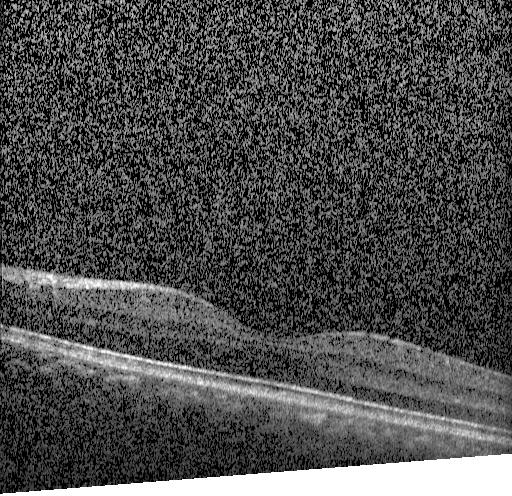
OCT finding: no choroidal neovascularization, diabetic macular edema, or drusen.